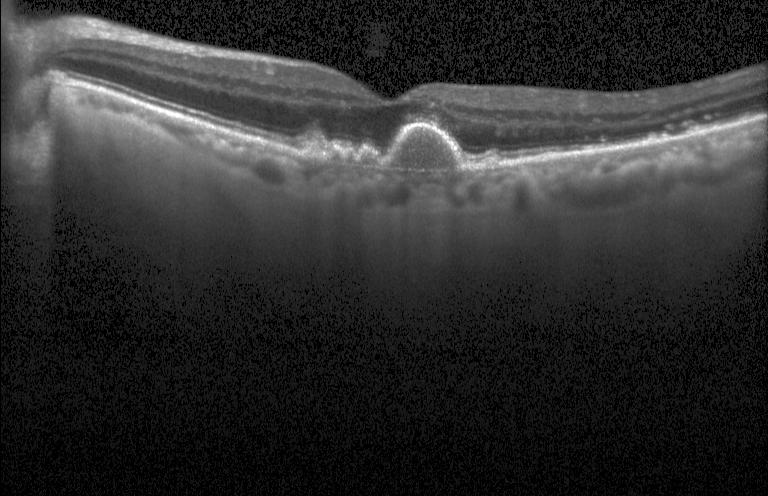

Impression: sub-RPE drusenoid deposits.